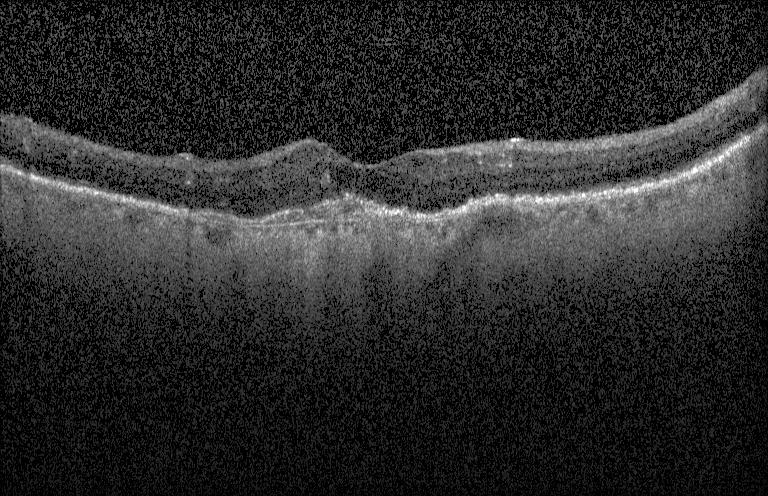

This B-scan demonstrates a choroidal neovascular membrane.